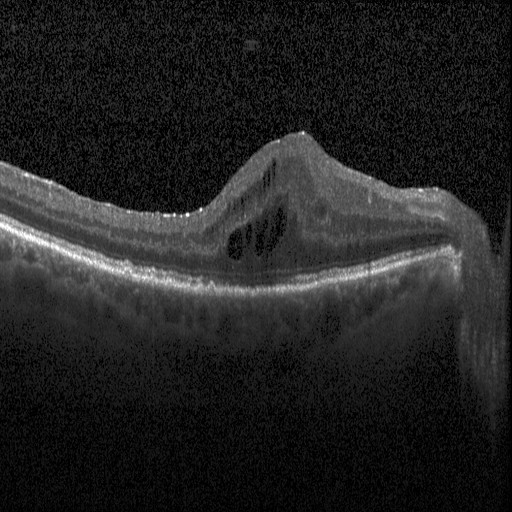

Retinal OCT B-scan. Through the macula. Spectral-domain OCT. Acquired on a Heidelberg Spectralis
Finding: diabetic macular edema (DME).